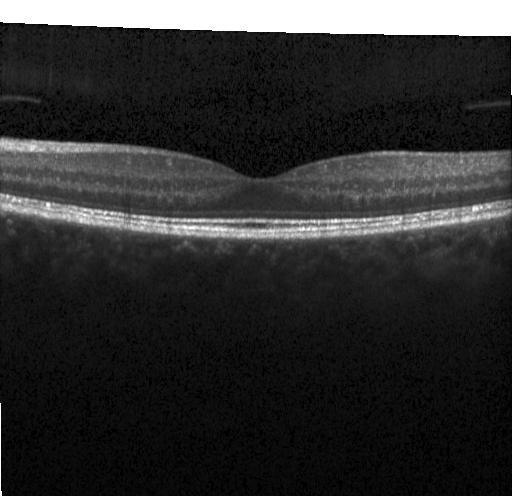

OCT B-scan showing no choroidal neovascularization, diabetic macular edema, or drusen.